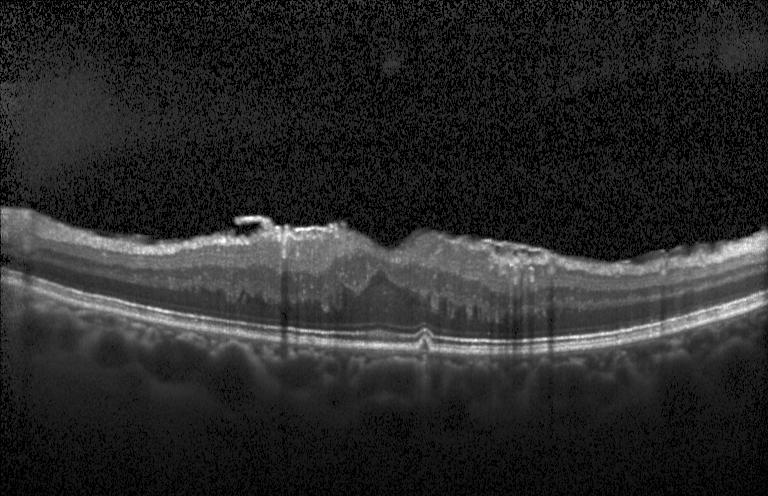
Macular OCT: sub-RPE drusenoid deposits.